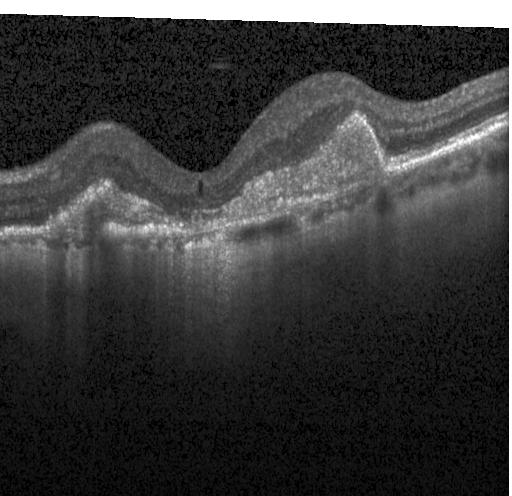
OCT B-scan; fovea-centered; Heidelberg Spectralis OCT system; spectral-domain optical coherence tomography. Finding: a choroidal neovascular membrane.